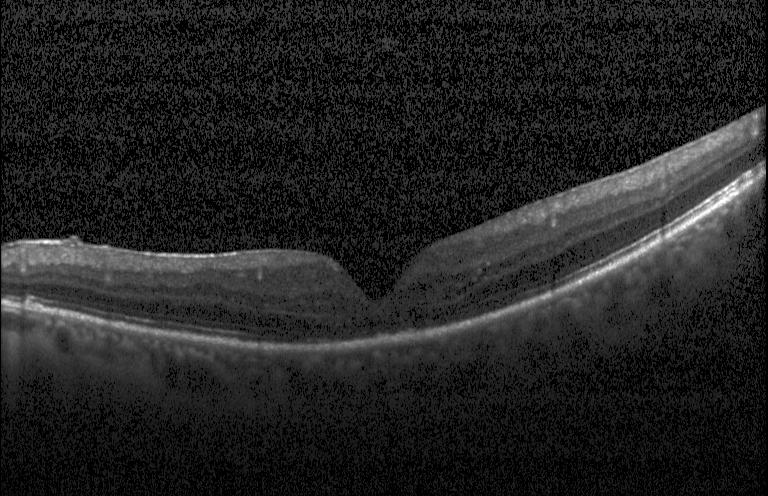

Instrument: Heidelberg Spectralis; optical coherence tomography scan.
Assessment: diabetic macular edema.